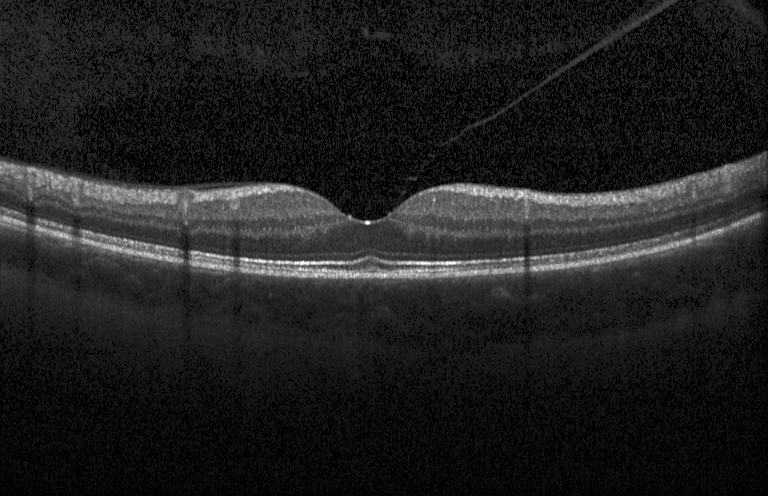 Impression: no choroidal neovascularization, no diabetic macular edema, and no drusen.